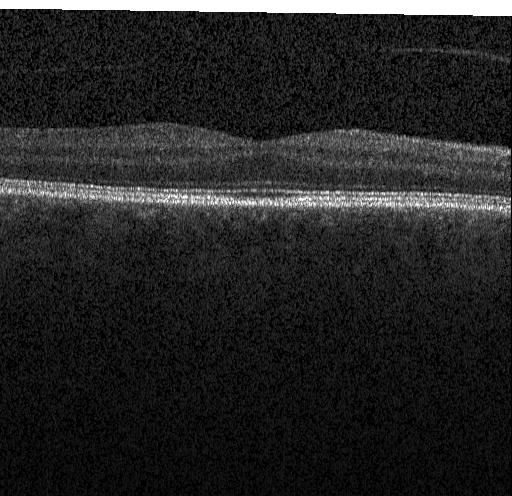
OCT B-scan — Impression: no CNV, DME, or drusen.